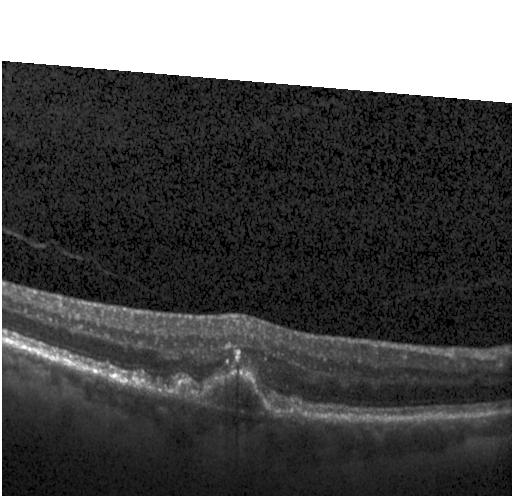

Retinal OCT B-scan
A choroidal neovascular membrane.